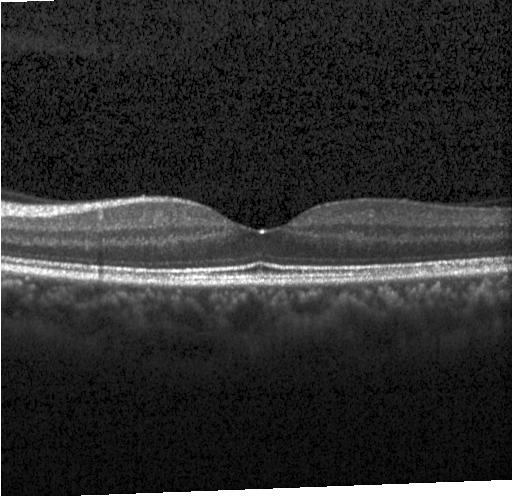 Macular scan, spectral-domain optical coherence tomography, retinal OCT B-scan, Heidelberg Spectralis OCT system.
Impression: neither choroidal neovascularization, diabetic macular edema, nor drusen.